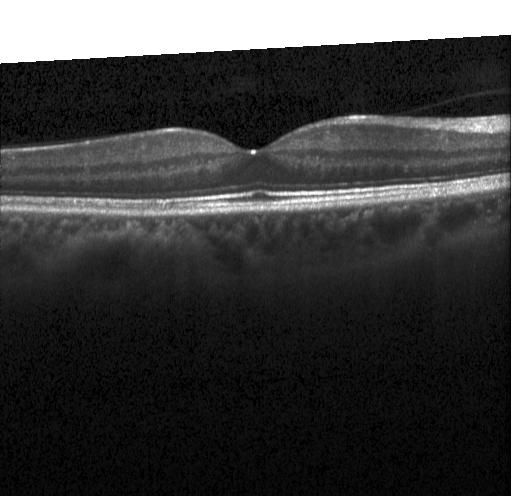
OCT line scan. This B-scan demonstrates no evidence of CNV, DME, or drusen.